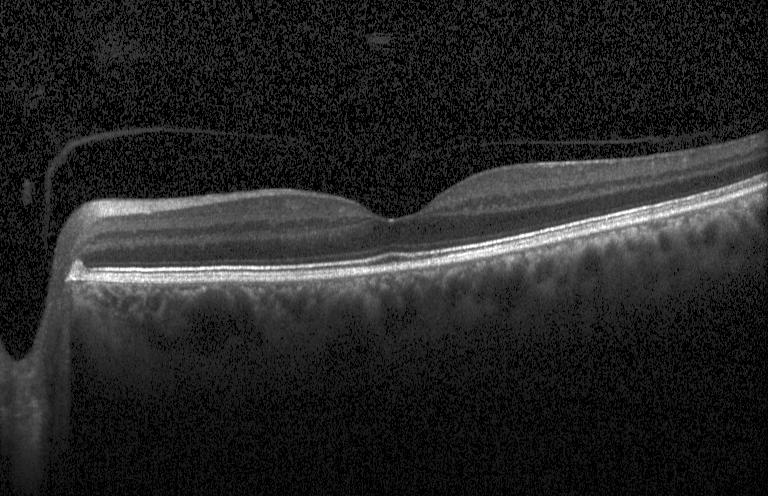

OCT line scan. Instrument: Heidelberg Spectralis. Fovea-centered. Spectral-domain optical coherence tomography.
Dx: no choroidal neovascularization, no diabetic macular edema, and no drusen.